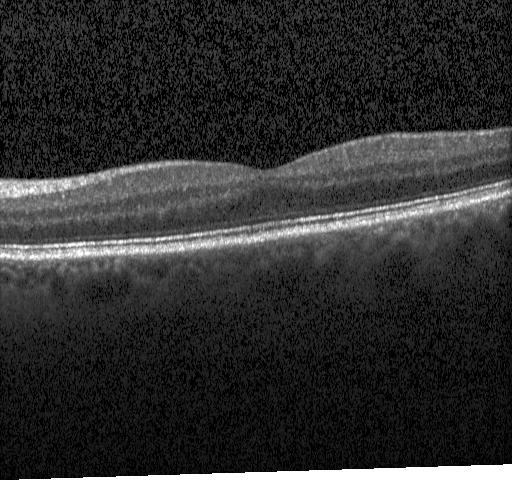

Optical coherence tomography B-scan
Assessment: neither choroidal neovascularization, diabetic macular edema, nor drusen.